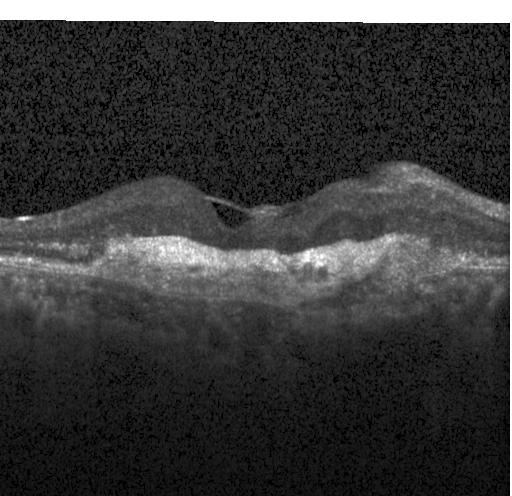
A choroidal neovascular membrane.